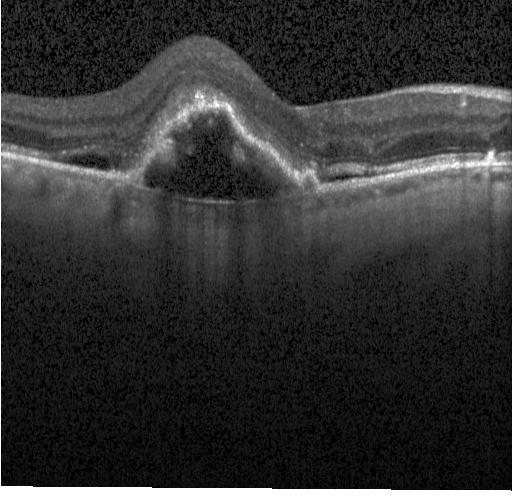

Acquired on a Heidelberg Spectralis; centered on the fovea; SD-OCT; optical coherence tomography B-scan. Diagnosis: CNV.